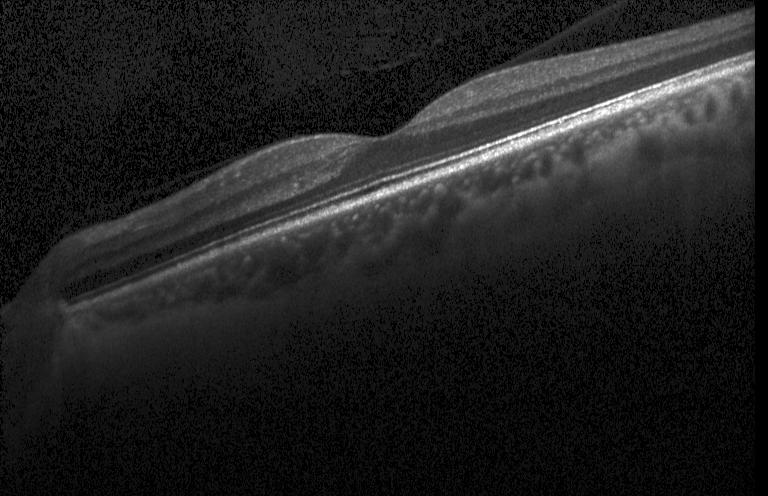 Macular OCT: neither choroidal neovascularization, diabetic macular edema, nor drusen.